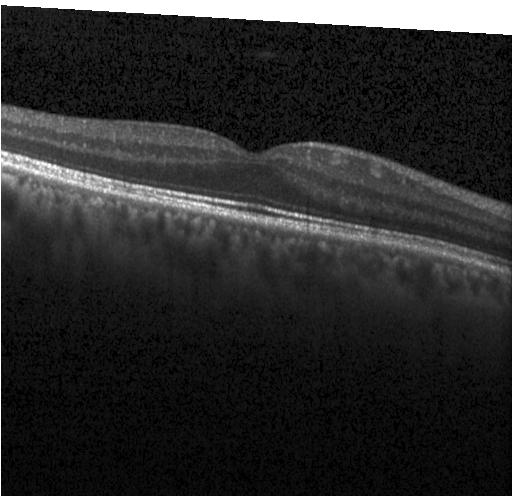
Optical coherence tomography B-scan. Assessment: no evidence of choroidal neovascularization, diabetic macular edema, or drusen.